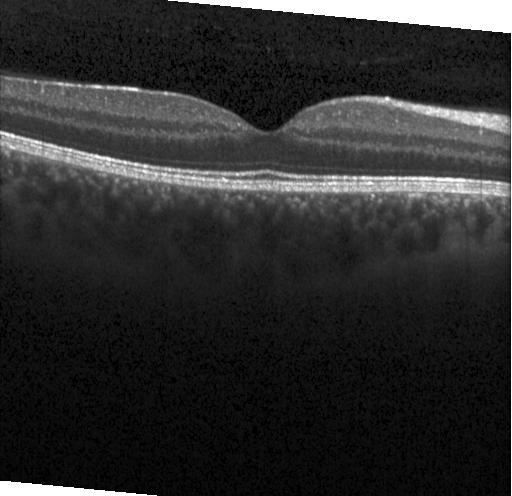

Finding: no CNV, no DME, and no drusen.